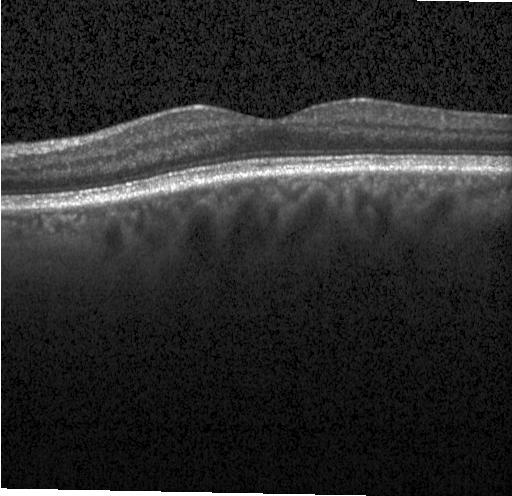 This B-scan demonstrates no choroidal neovascularization, no diabetic macular edema, and no drusen.